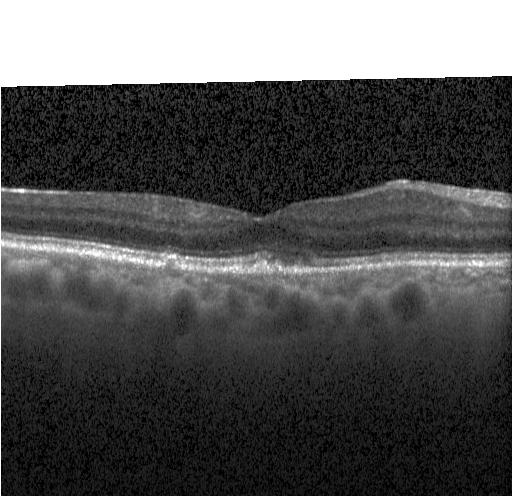
Retinal OCT cross-section; macular scan; spectral-domain optical coherence tomography.
The scan shows drusen.